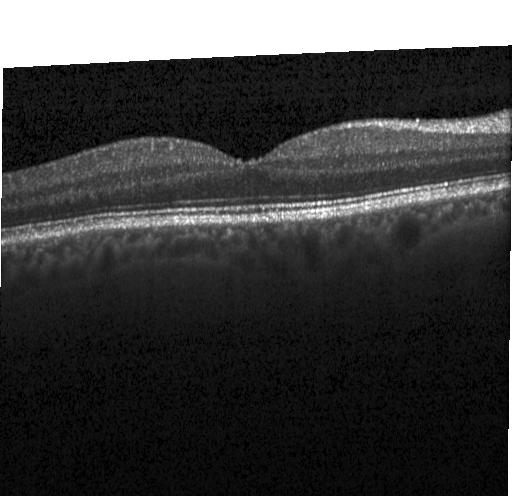

Optical coherence tomography B-scan
Diagnosis: no choroidal neovascularization, no diabetic macular edema, and no drusen.